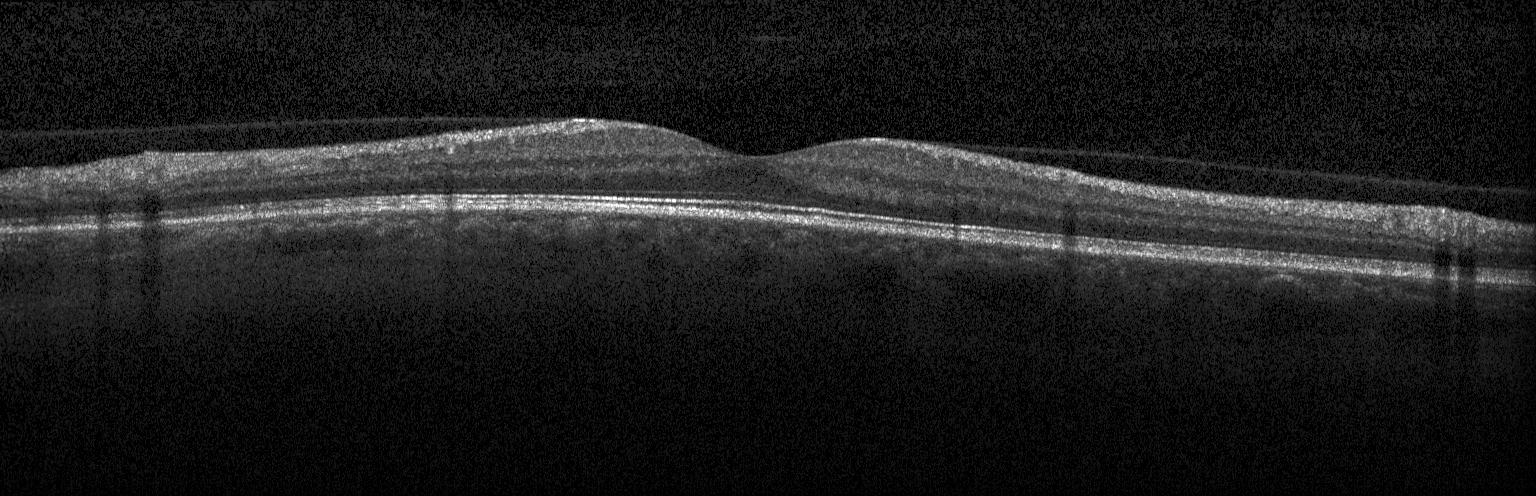

OCT line scan
The scan shows neither choroidal neovascularization, diabetic macular edema, nor drusen.